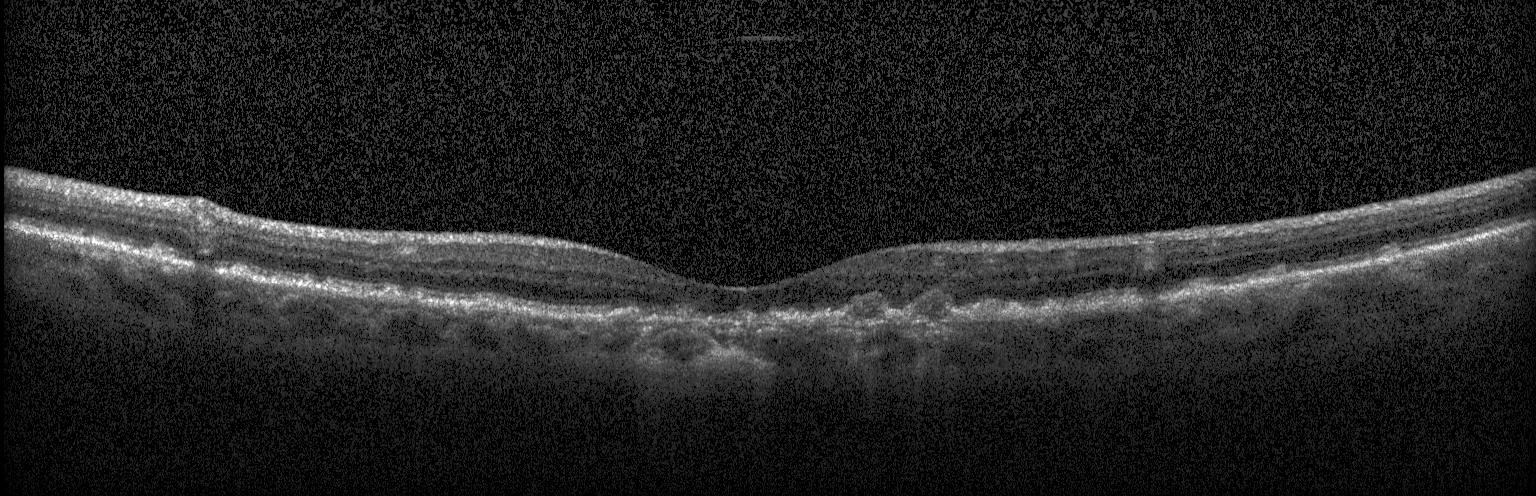
Optical coherence tomography scan. Heidelberg Spectralis OCT system. This B-scan demonstrates a choroidal neovascular membrane.